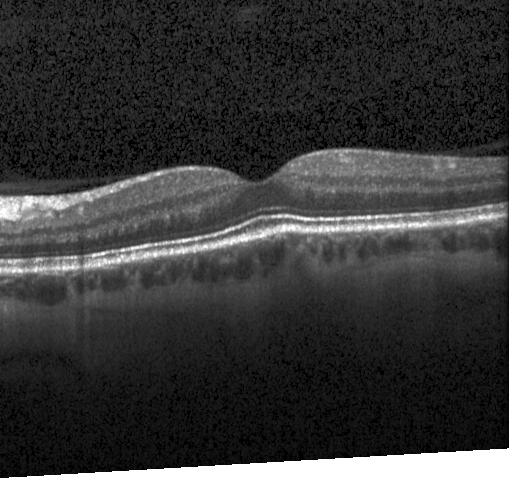
Optical coherence tomography scan · acquired on a Heidelberg Spectralis
Finding: no evidence of choroidal neovascularization, diabetic macular edema, or drusen.